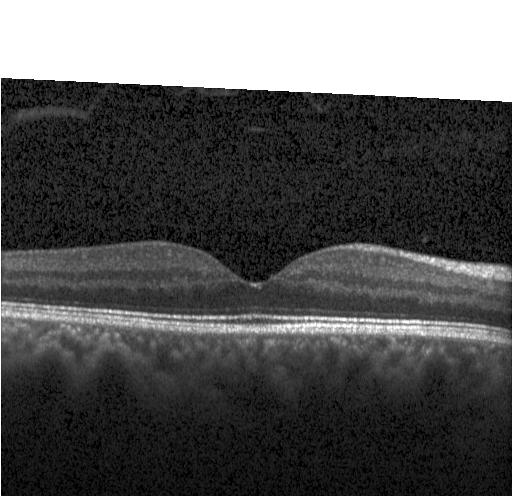
Optical coherence tomography B-scan.
Assessment: no choroidal neovascularization, diabetic macular edema, or drusen.